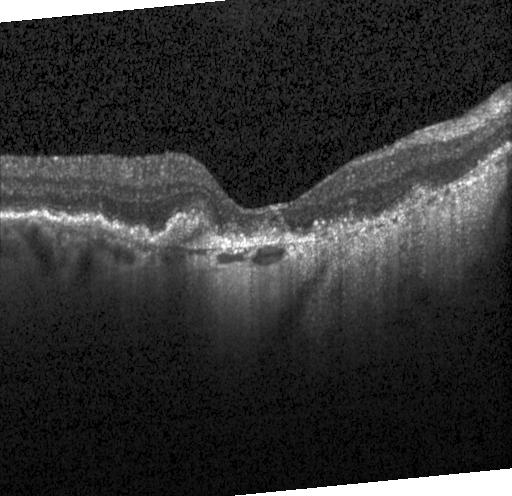

Retinal OCT B-scan; SD-OCT; through the macula. Impression: choroidal neovascularization (CNV).